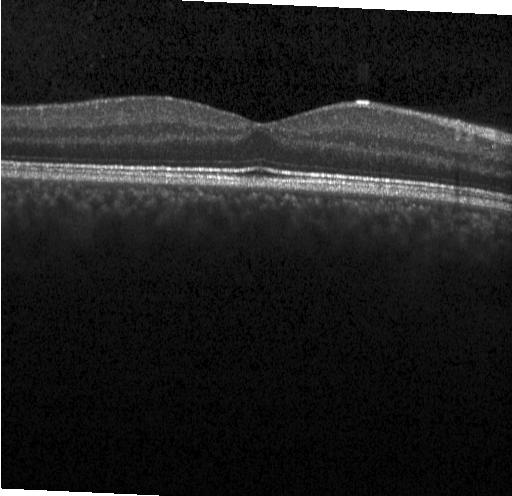
Retinal OCT B-scan, Heidelberg Spectralis OCT system. No evidence of choroidal neovascularization, diabetic macular edema, or drusen.